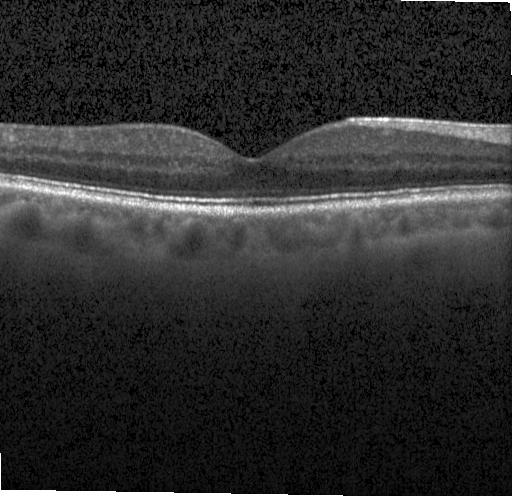

No CNV, DME, or drusen.